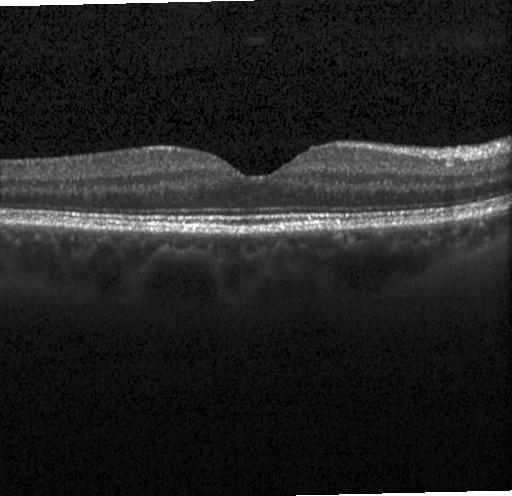

OCT B-scan. Centered on the fovea. SD-OCT. Dx: no evidence of CNV, DME, or drusen.